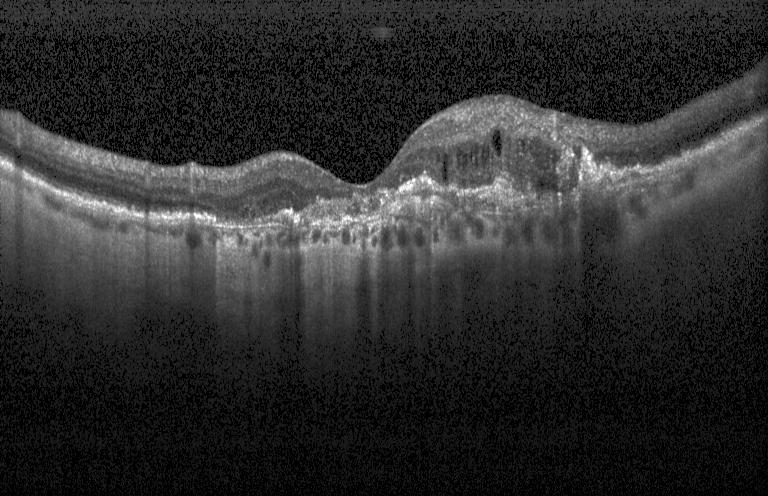
Macular OCT: choroidal neovascularization.